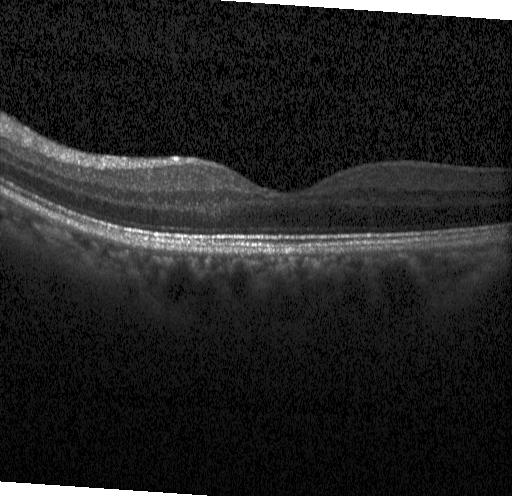
Fovea-centered, OCT line scan
Assessment: no choroidal neovascularization, diabetic macular edema, or drusen.